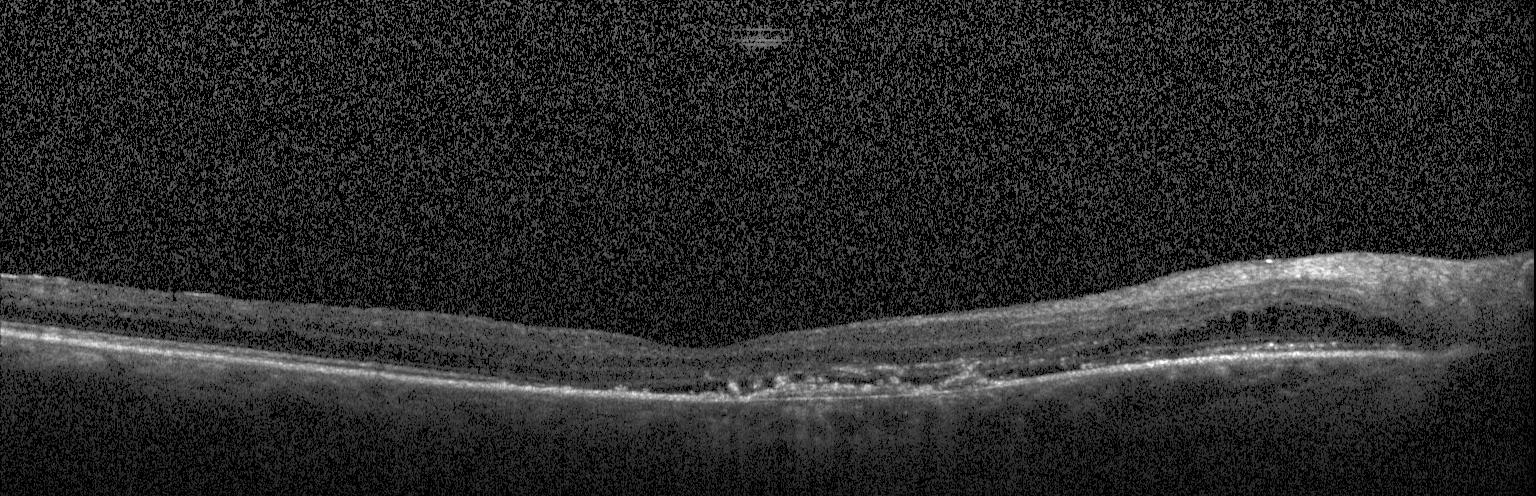

OCT B-scan; instrument: Heidelberg Spectralis
Impression: choroidal neovascularization (CNV).